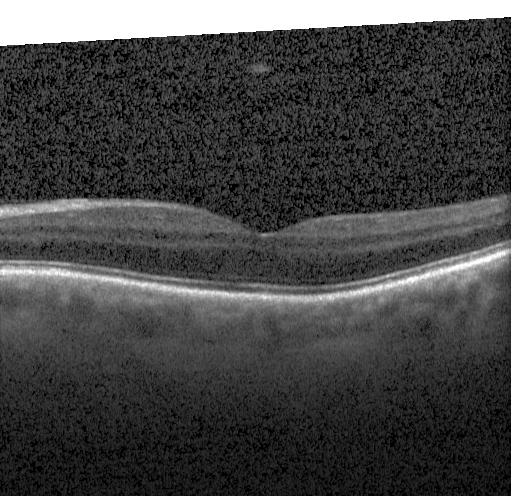

Fovea-centered · Heidelberg Spectralis · optical coherence tomography B-scan · spectral-domain optical coherence tomography. Impression: no choroidal neovascularization, diabetic macular edema, or drusen.